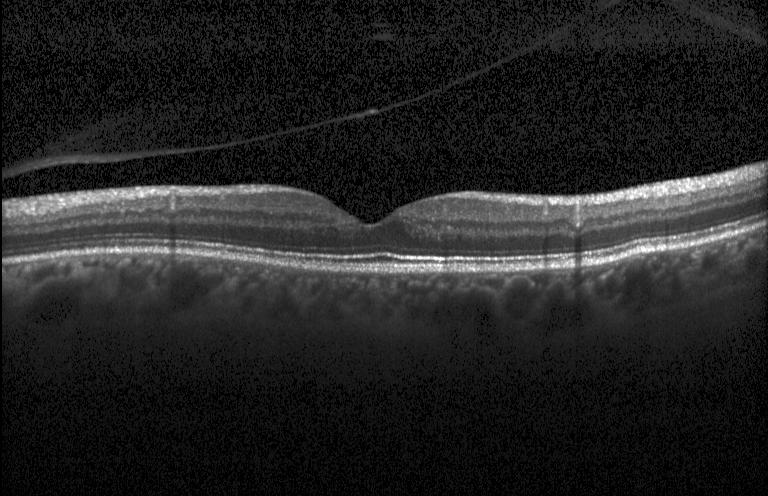

Horizontal scan through the fovea, SD-OCT, optical coherence tomography B-scan
Macular OCT: neither CNV, DME, nor drusen.